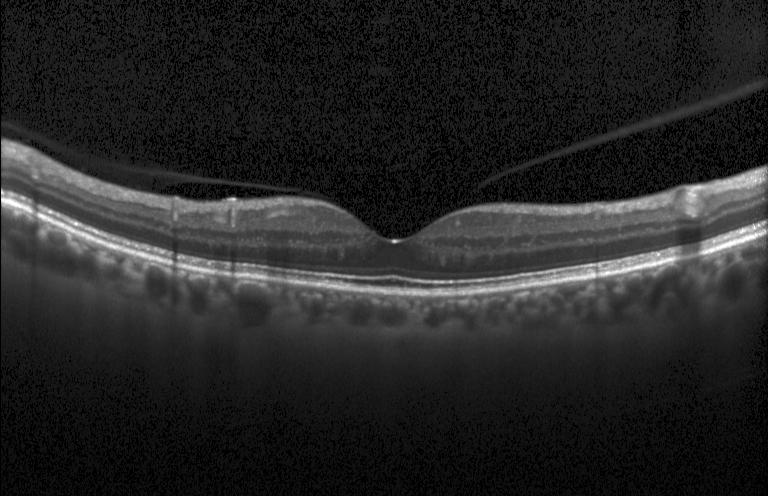 Impression: no CNV, no DME, and no drusen.